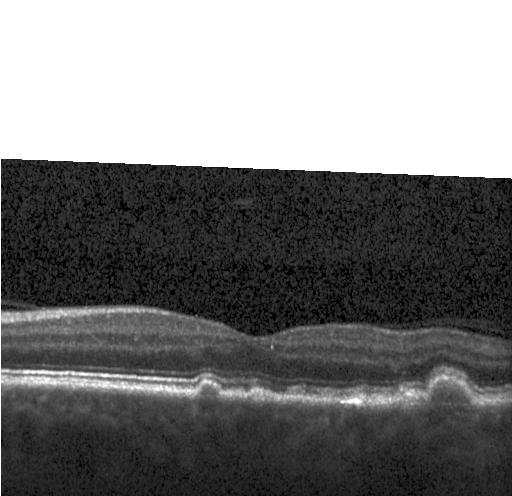

OCT line scan — Macular OCT: drusen.